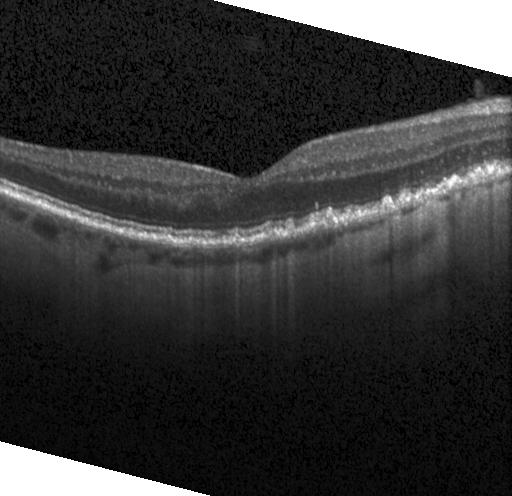 Diagnosis: sub-RPE drusenoid deposits.